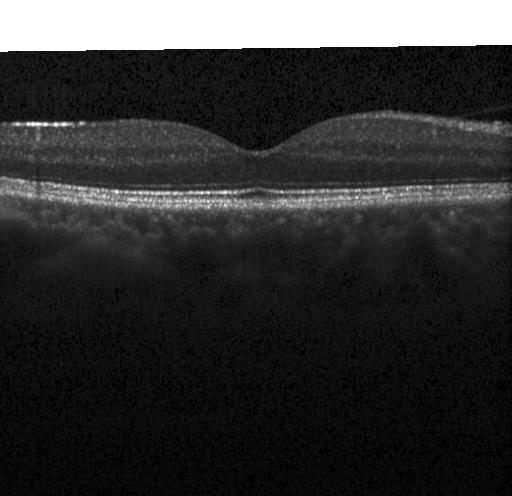

Optical coherence tomography scan · SD-OCT — Finding: neither choroidal neovascularization, diabetic macular edema, nor drusen.